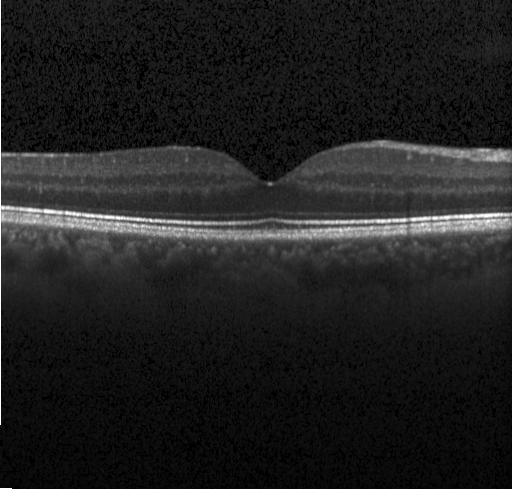
Optical coherence tomography scan.
Impression: no evidence of CNV, DME, or drusen.